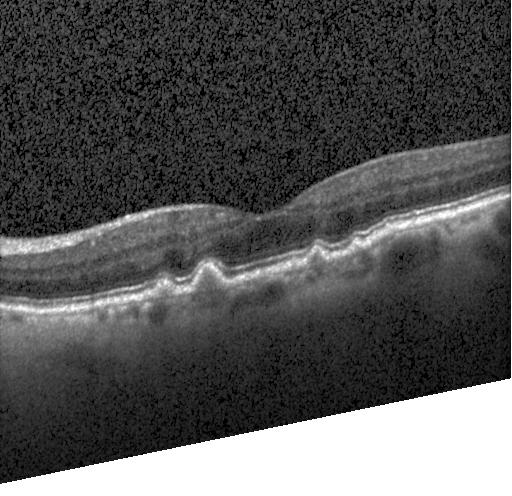

Finding: multiple drusen.